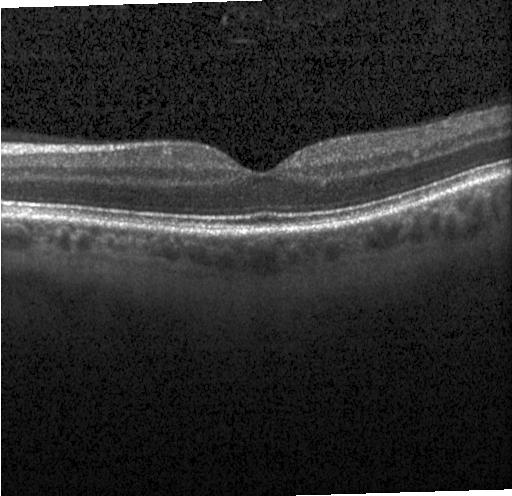 No evidence of choroidal neovascularization, diabetic macular edema, or drusen.